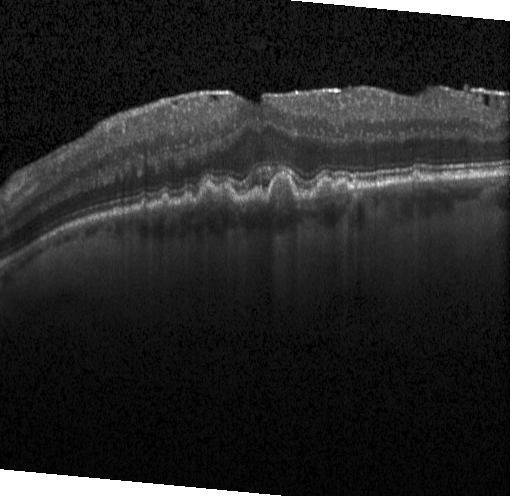

Impression: drusen.